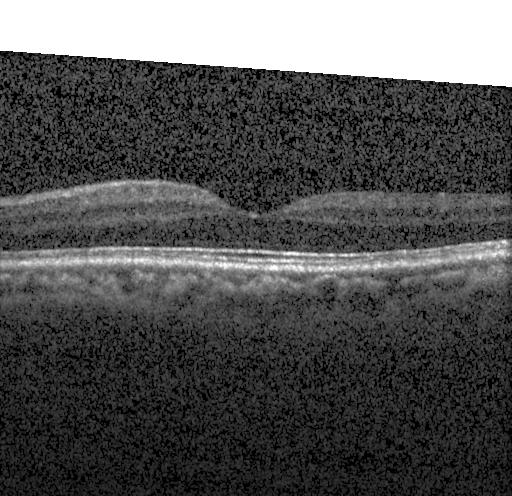

Heidelberg Spectralis OCT system, macular scan, retinal OCT cross-section
Assessment: no evidence of CNV, DME, or drusen.